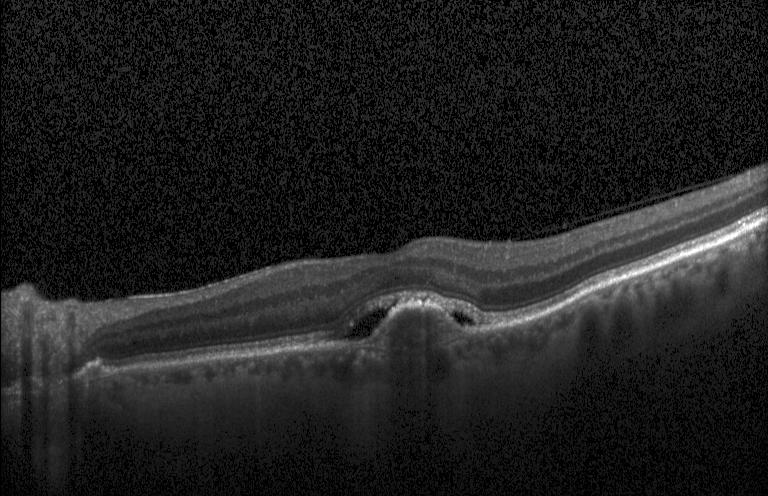 OCT line scan.
Dx: a choroidal neovascular membrane.